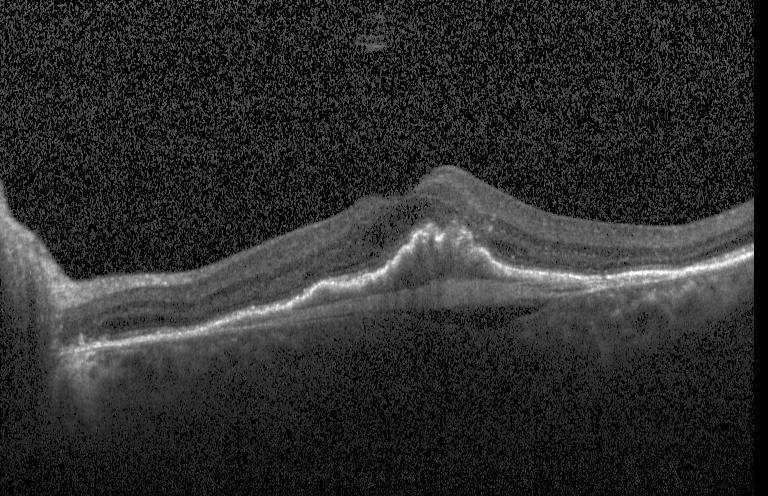
Optical coherence tomography scan, through the macula, SD-OCT — Impression: CNV.